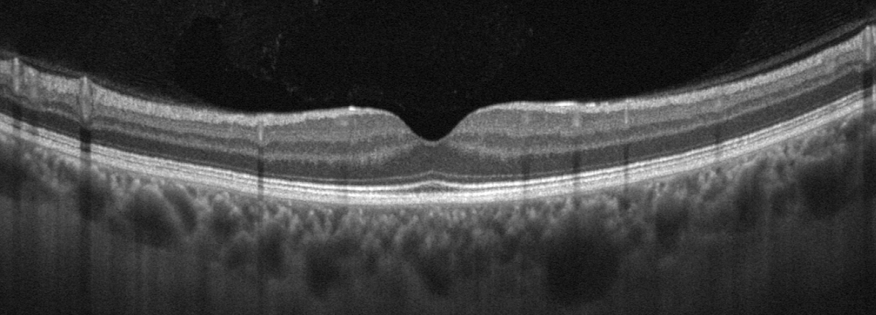

Optovue Avanti RTVue XR; retinal OCT cross-section.
Finding: no AMD, DME, ERM, RAO, RVO, or VID.